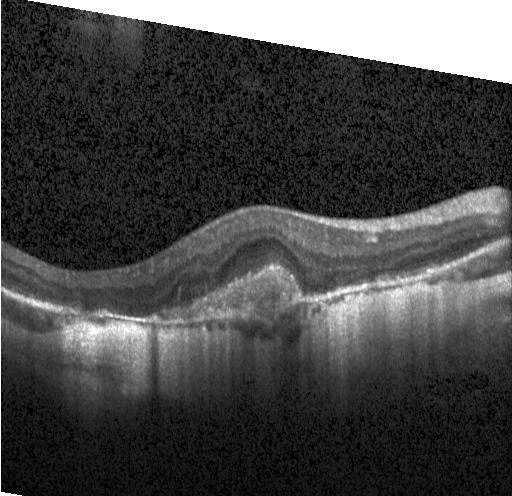
Impression: a choroidal neovascular membrane.